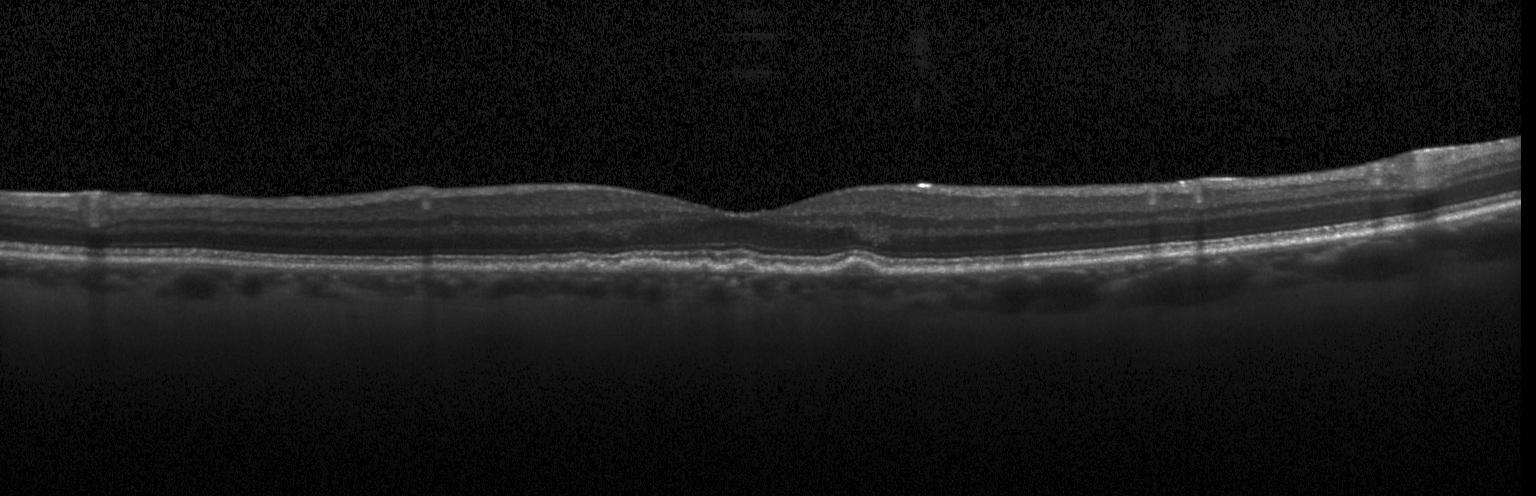
Through the macula, OCT B-scan, spectral-domain OCT, Heidelberg Spectralis OCT system. Assessment: sub-RPE drusenoid deposits.